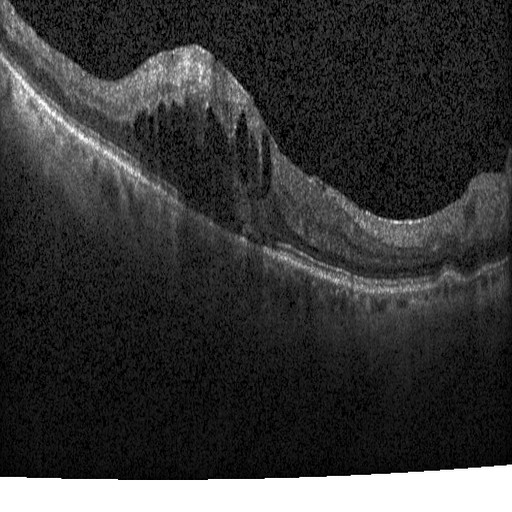 Fovea-centered; spectral-domain optical coherence tomography; Heidelberg Spectralis OCT system; retinal OCT cross-section — Finding: diabetic macular edema.